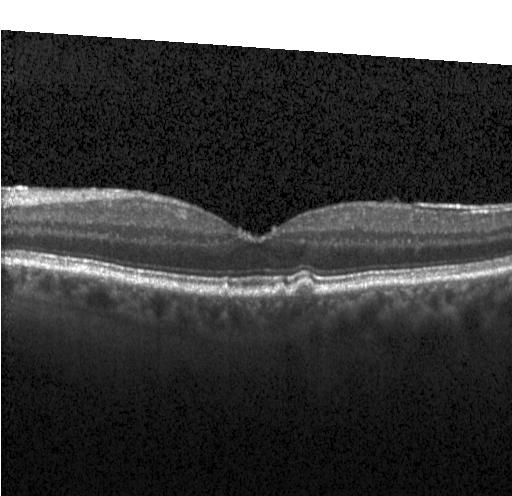
Through the macula, acquired on a Heidelberg Spectralis, OCT line scan, spectral-domain OCT. Macular OCT: sub-RPE drusenoid deposits.